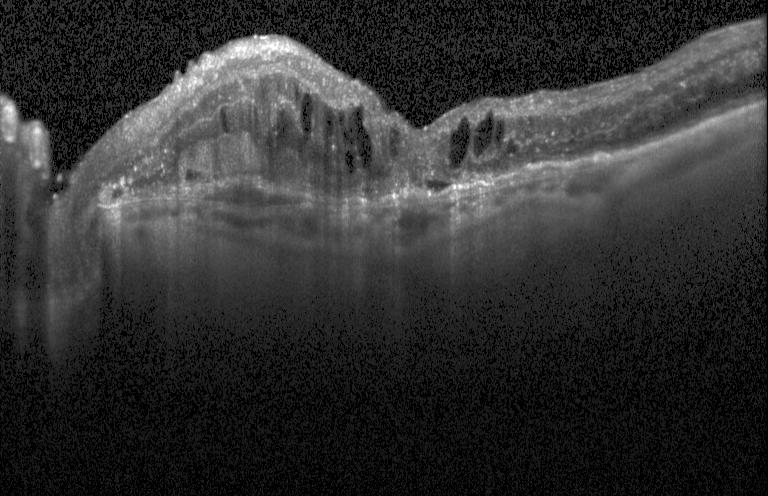 Acquired on a Heidelberg Spectralis. Macular scan. Retinal OCT cross-section
Dx: CNV.